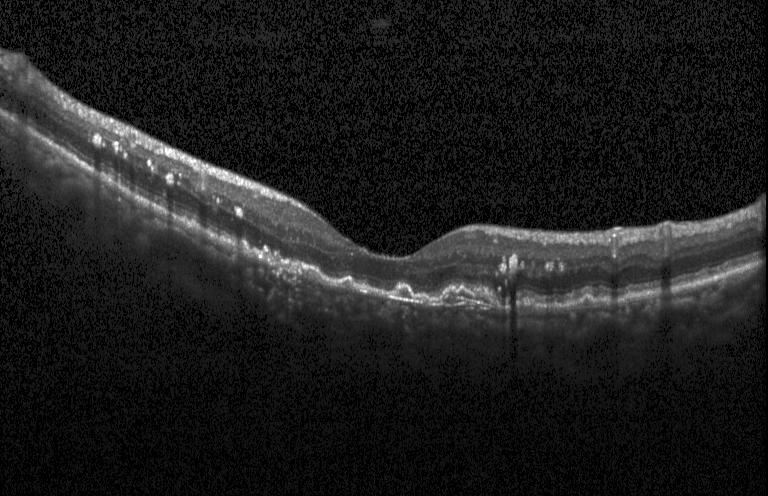
Optical coherence tomography scan
Finding: a choroidal neovascular membrane.